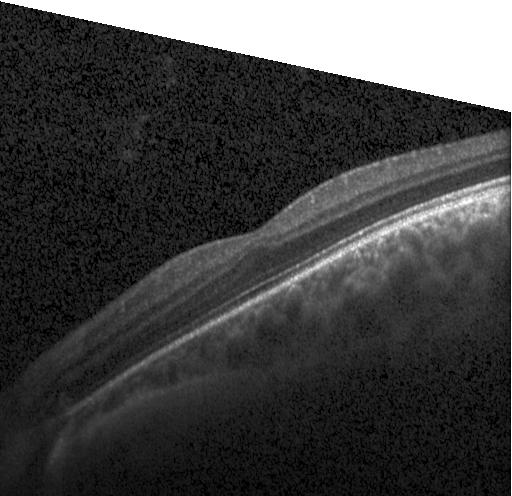 OCT B-scan
Macular OCT: neither choroidal neovascularization, diabetic macular edema, nor drusen.